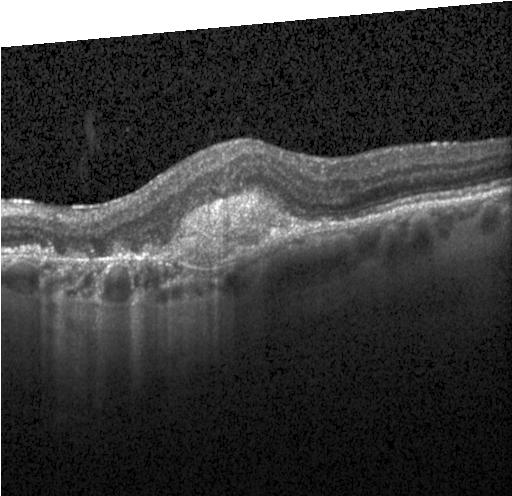 Retinal OCT B-scan, centered on the fovea, Heidelberg Spectralis, spectral-domain OCT.
Diagnosis: choroidal neovascularization.